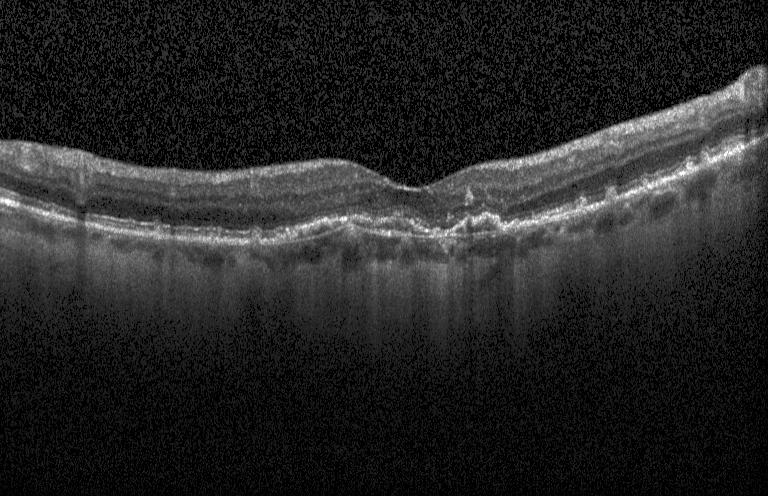 Heidelberg Spectralis OCT system · horizontal scan through the fovea · spectral-domain optical coherence tomography · optical coherence tomography B-scan — Assessment: choroidal neovascularization.